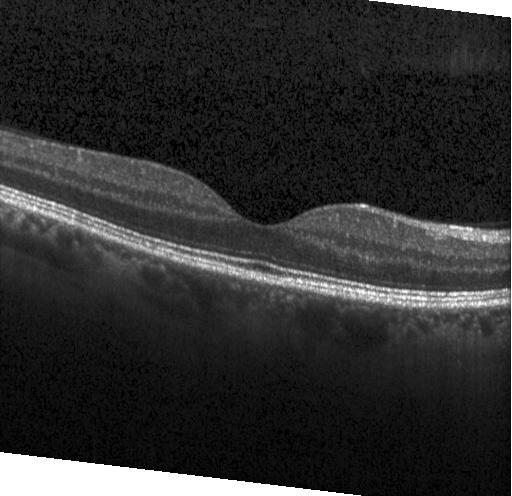

Macular scan · retinal OCT cross-section — No evidence of choroidal neovascularization, diabetic macular edema, or drusen.